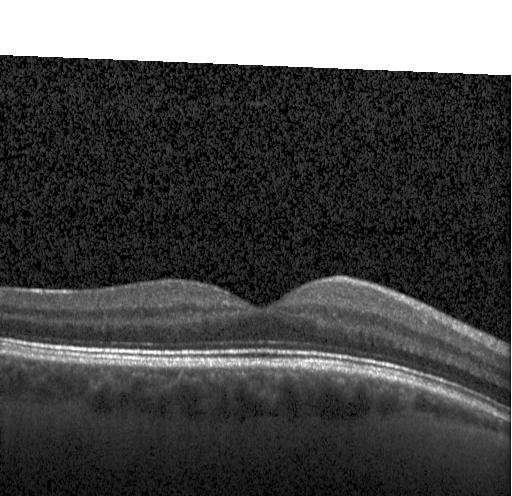

Impression: neither choroidal neovascularization, diabetic macular edema, nor drusen.